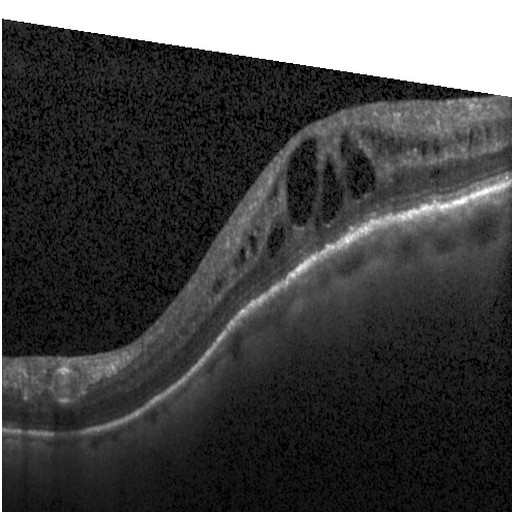

Optical coherence tomography scan · macular scan · SD-OCT · Heidelberg Spectralis
Diagnosis: diabetic macular edema.